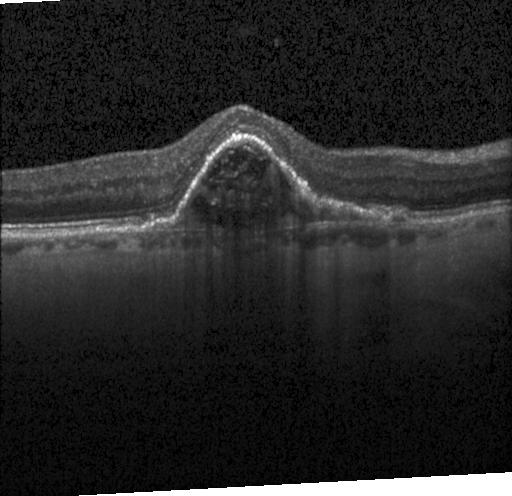 This B-scan demonstrates CNV.